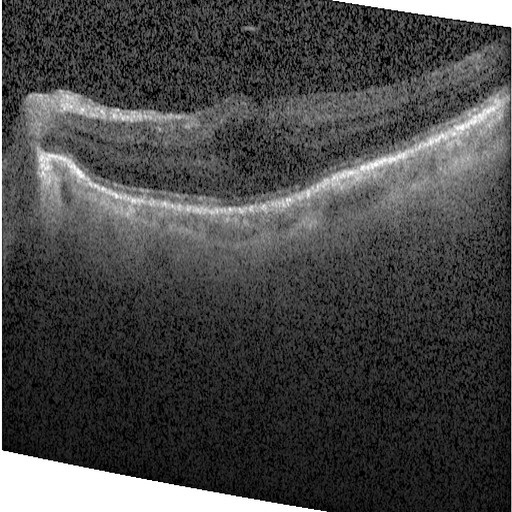

Retinal OCT cross-section — Assessment: diabetic macular edema.